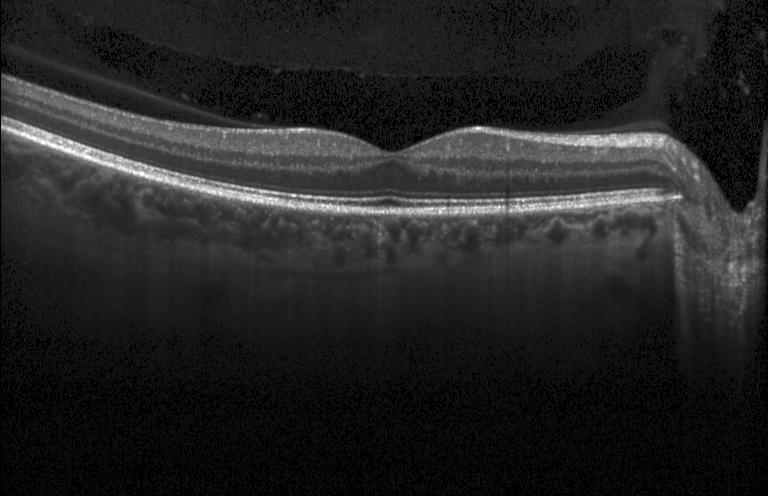
The scan shows no choroidal neovascularization, no diabetic macular edema, and no drusen.